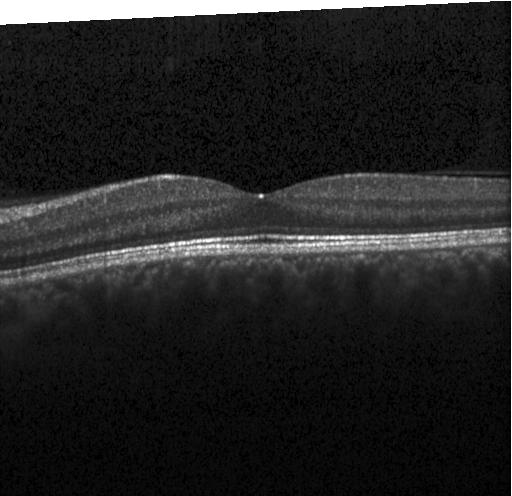 Dx: neither choroidal neovascularization, diabetic macular edema, nor drusen.